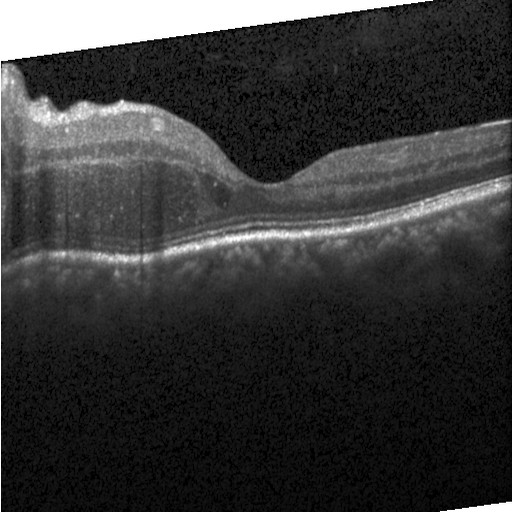

Spectral-domain OCT, OCT B-scan, macular scan, acquired on a Heidelberg Spectralis
Assessment: diabetic macular edema (DME).